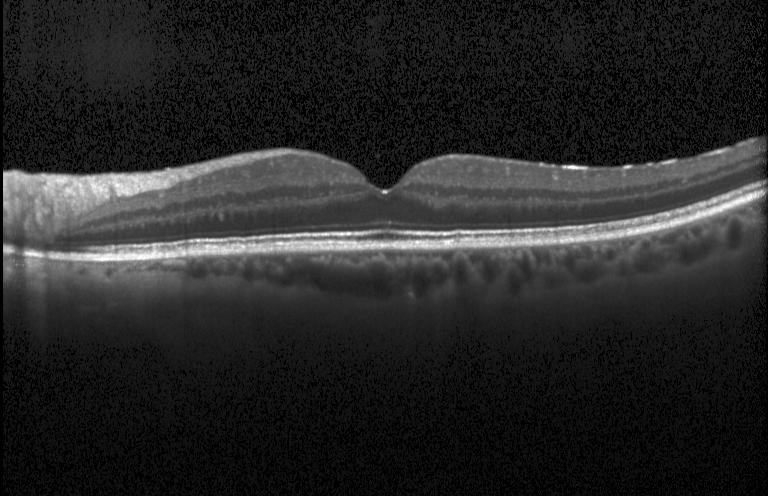 OCT B-scan.
Diagnosis: neither choroidal neovascularization, diabetic macular edema, nor drusen.